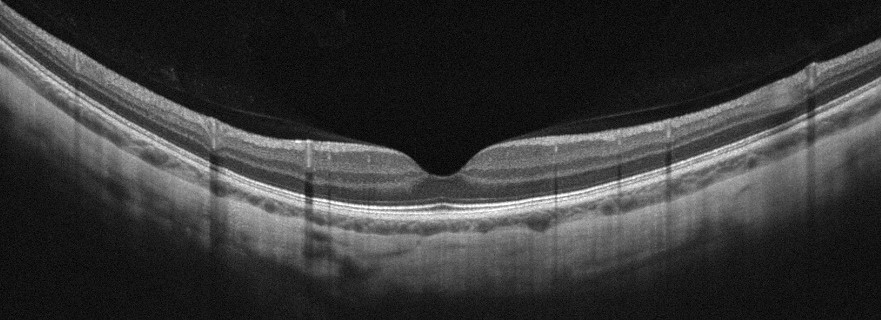
OCT B-scan, fovea-centered, acquired on an Optovue Avanti RTVue XR. Assessment: absence of AMD, DME, ERM, RAO, RVO, and vitreomacular interface disease.